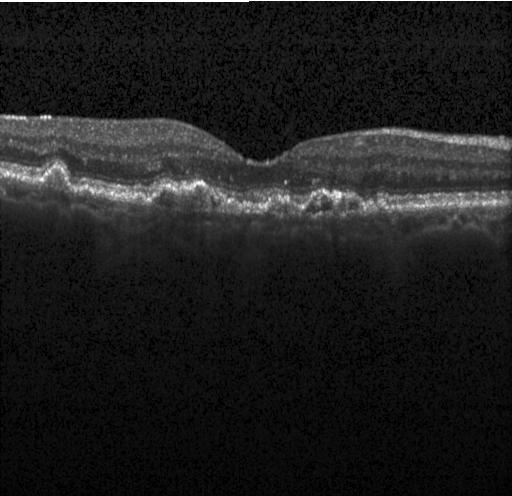 Through the macula; spectral-domain optical coherence tomography; optical coherence tomography scan; instrument: Heidelberg Spectralis. Impression: a choroidal neovascular membrane.